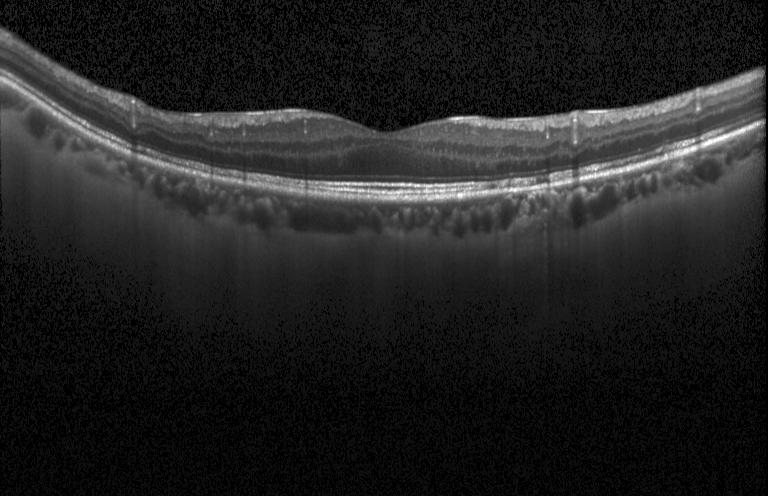

Optical coherence tomography B-scan
Finding: no evidence of choroidal neovascularization, diabetic macular edema, or drusen.